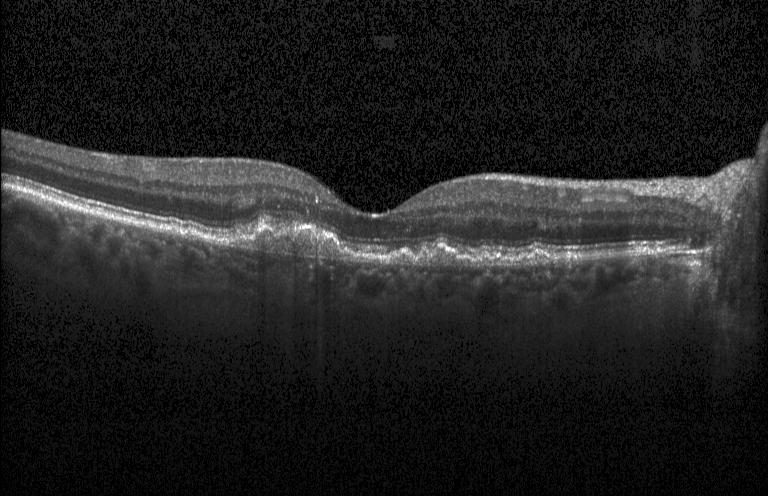

OCT finding: choroidal neovascularization.